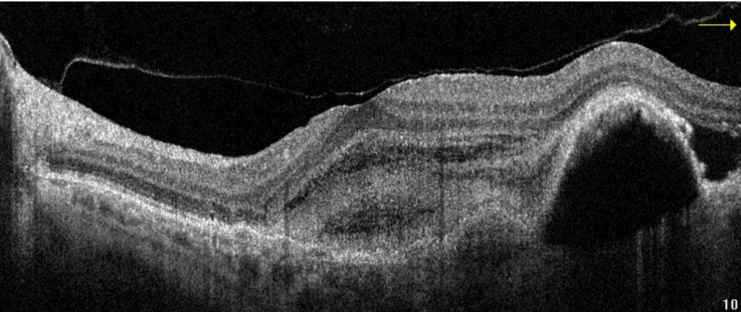
OCT B-scan · acquired on an Optovue Avanti RTVue XR · macular scan. Finding: age-related macular degeneration (AMD).